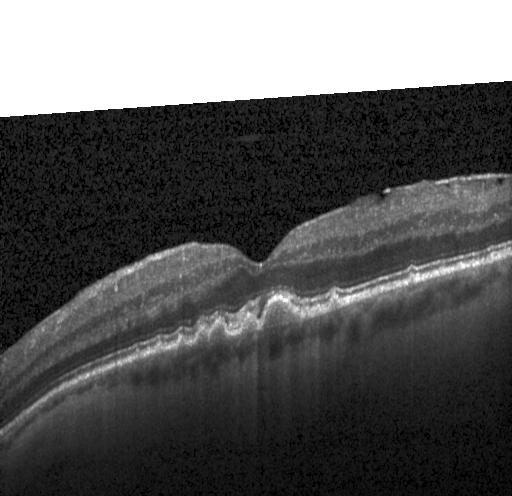

Horizontal scan through the fovea; retinal OCT B-scan. OCT finding: drusen.